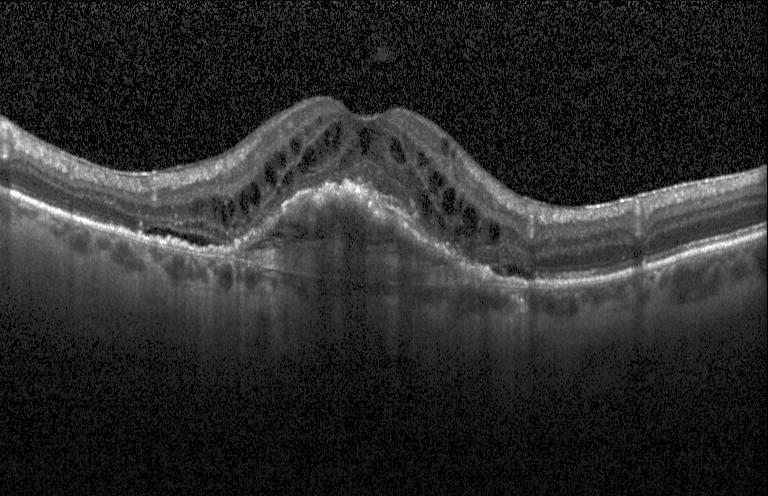
Retinal OCT B-scan.
Diagnosis: a choroidal neovascular membrane.